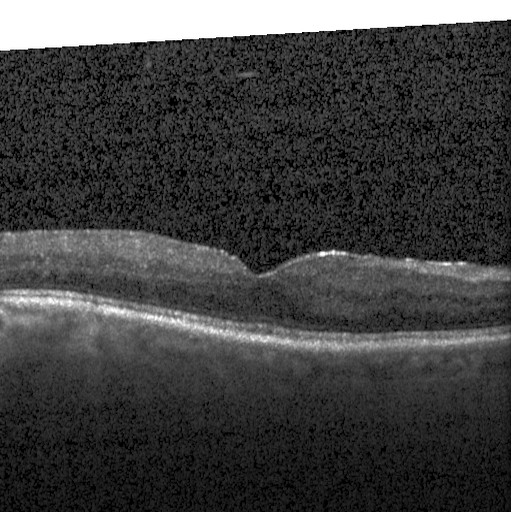

Through the macula; SD-OCT; retinal OCT B-scan; acquired on a Heidelberg Spectralis
Impression: diabetic macular edema.